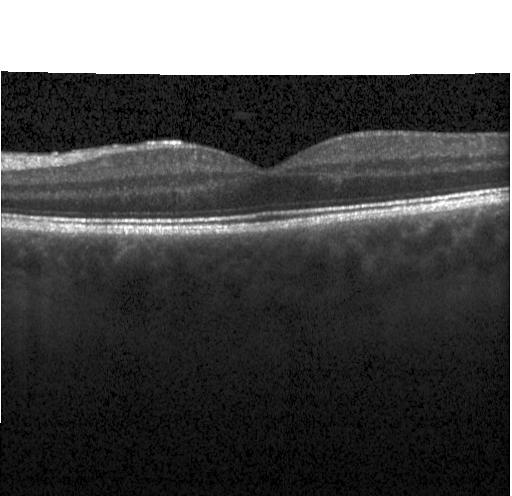

Impression: no choroidal neovascularization, no diabetic macular edema, and no drusen.